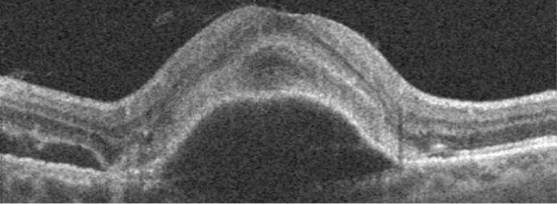

Retinal OCT cross-section — Finding: age-related macular degeneration (AMD).